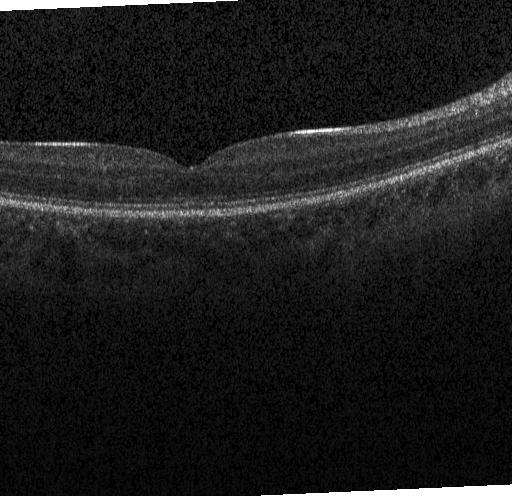
Diagnosis: neither choroidal neovascularization, diabetic macular edema, nor drusen.